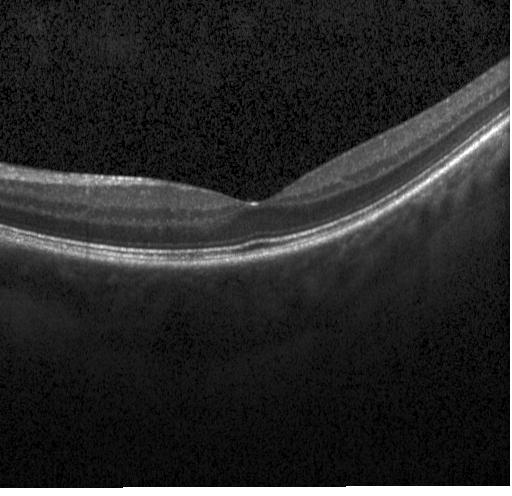
OCT B-scan. Diagnosis: neither CNV, DME, nor drusen.